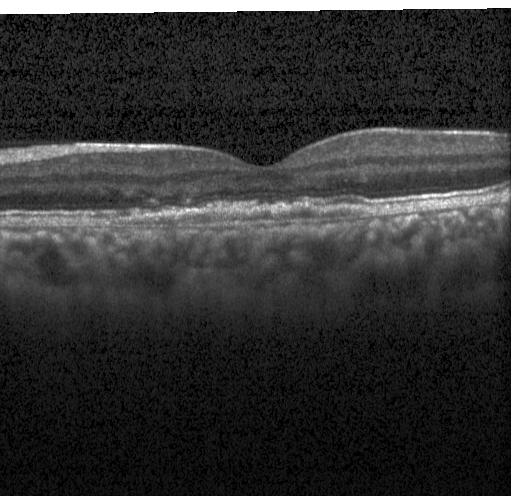

OCT B-scan; fovea-centered; SD-OCT.
The scan shows CNV.